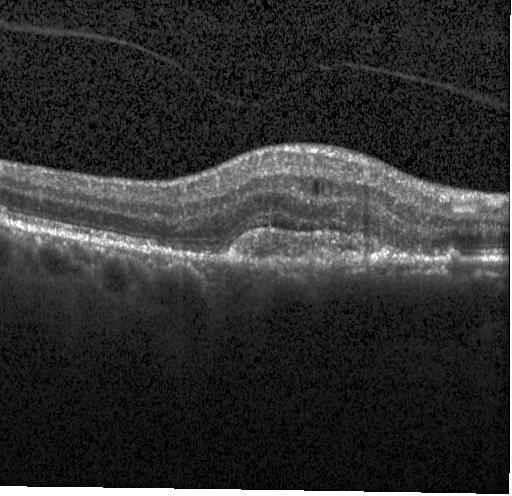
OCT line scan; spectral-domain optical coherence tomography; fovea-centered
Finding: choroidal neovascularization (CNV).